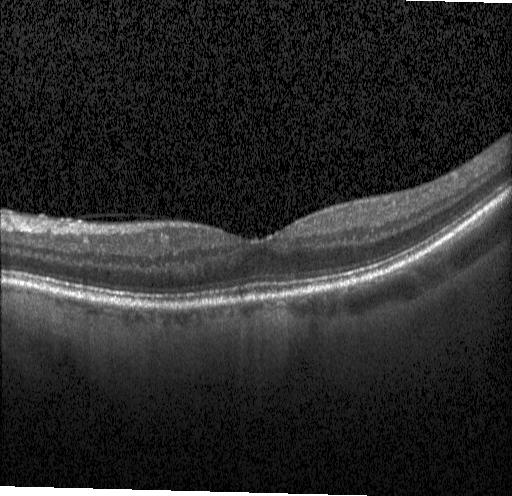

Diagnosis: neither CNV, DME, nor drusen.